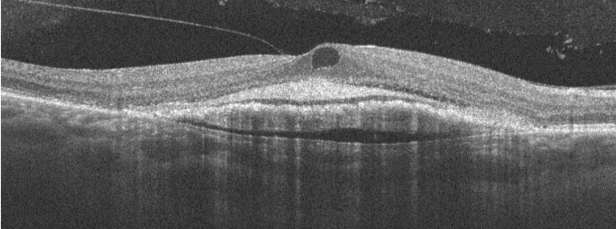 Age-related macular degeneration.